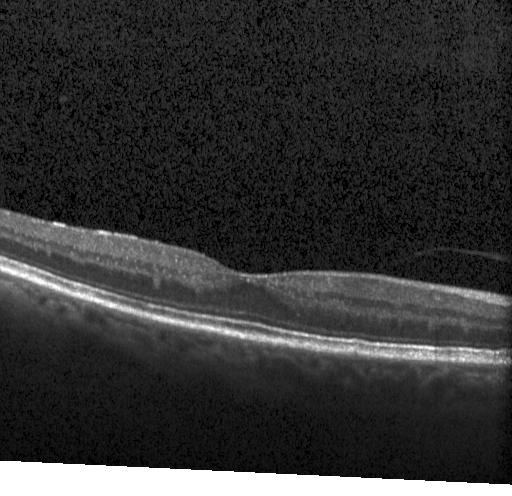 SD-OCT. Optical coherence tomography scan. Heidelberg Spectralis OCT system — This B-scan demonstrates no evidence of choroidal neovascularization, diabetic macular edema, or drusen.